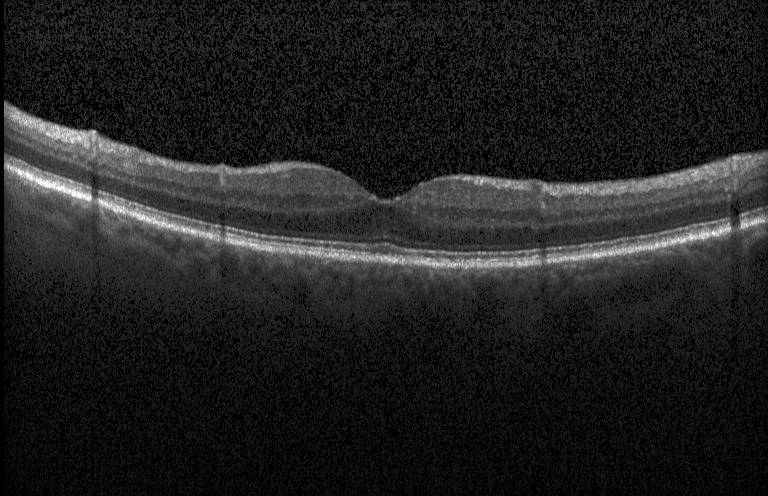

Optical coherence tomography B-scan — Finding: no choroidal neovascularization, diabetic macular edema, or drusen.